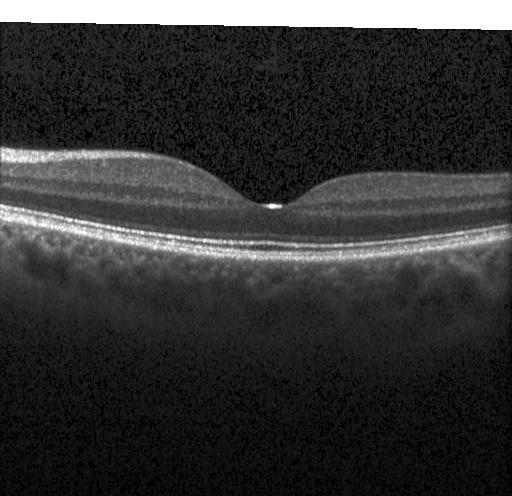 Retinal OCT B-scan
The scan shows no CNV, DME, or drusen.